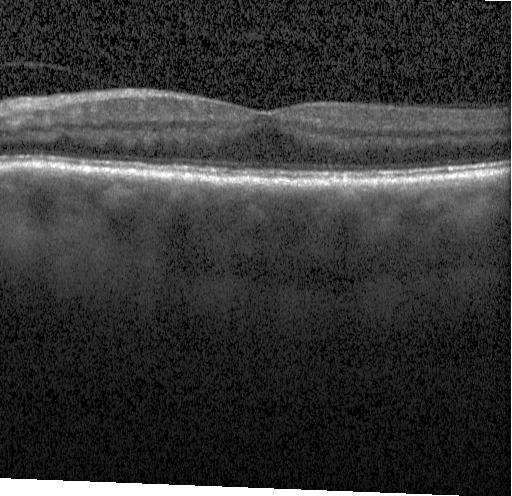

Neither choroidal neovascularization, diabetic macular edema, nor drusen.